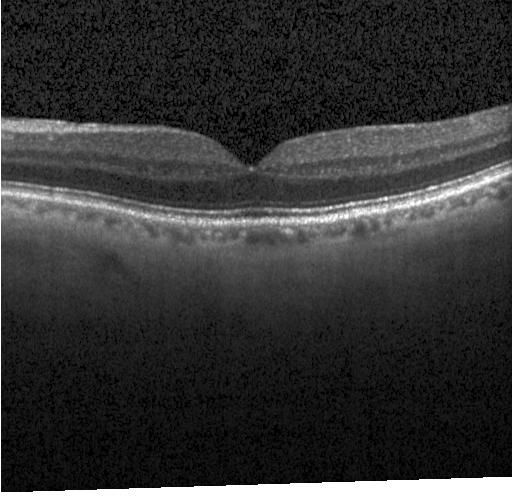

SD-OCT; centered on the fovea; instrument: Heidelberg Spectralis; OCT line scan. Impression: no choroidal neovascularization, no diabetic macular edema, and no drusen.